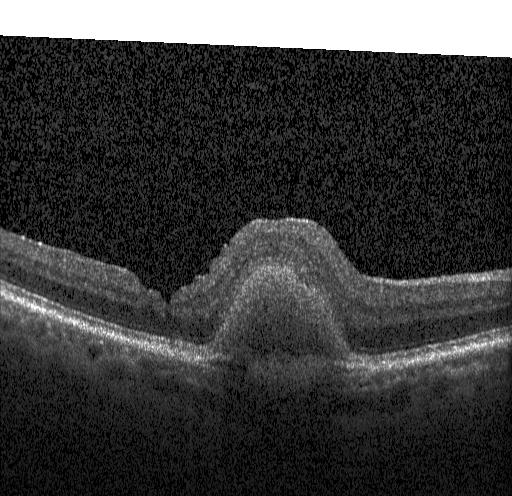
OCT line scan
Finding: a choroidal neovascular membrane.